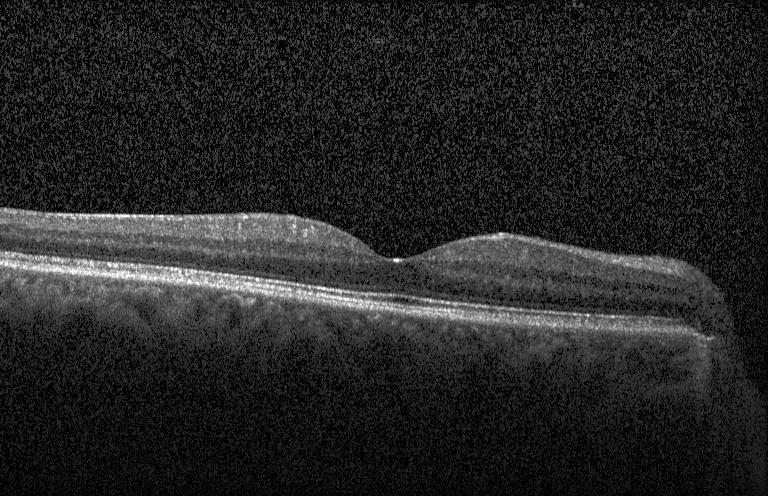
Retinal OCT B-scan · fovea-centered · SD-OCT · instrument: Heidelberg Spectralis — This B-scan demonstrates no CNV, no DME, and no drusen.